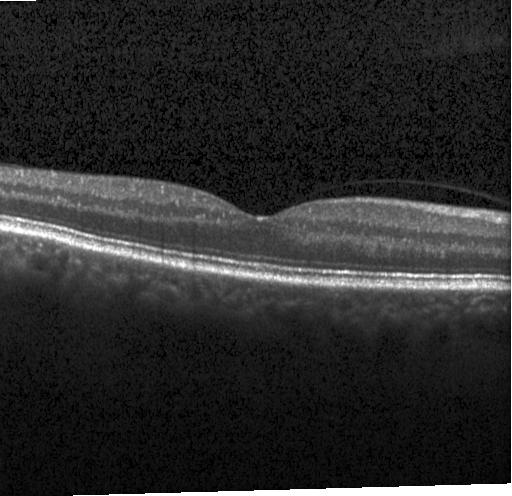 This B-scan demonstrates no choroidal neovascularization, no diabetic macular edema, and no drusen.